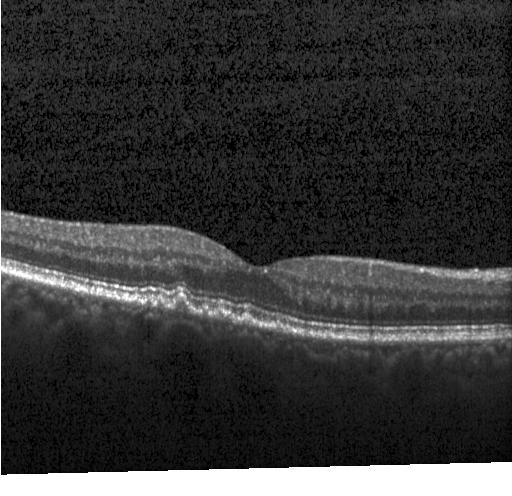
Retinal OCT B-scan.
Finding: drusen.